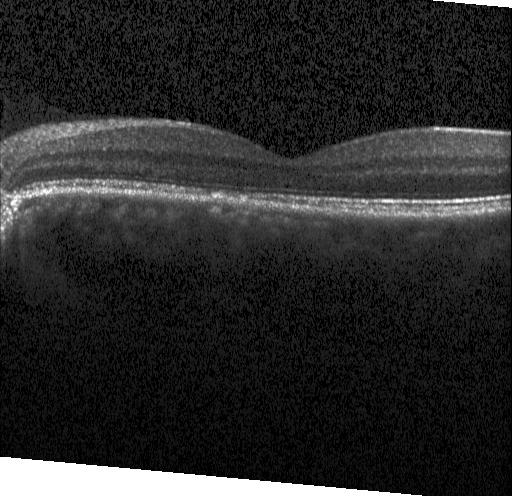
Instrument: Heidelberg Spectralis. Retinal OCT cross-section. Through the macula.
Finding: no evidence of choroidal neovascularization, diabetic macular edema, or drusen.